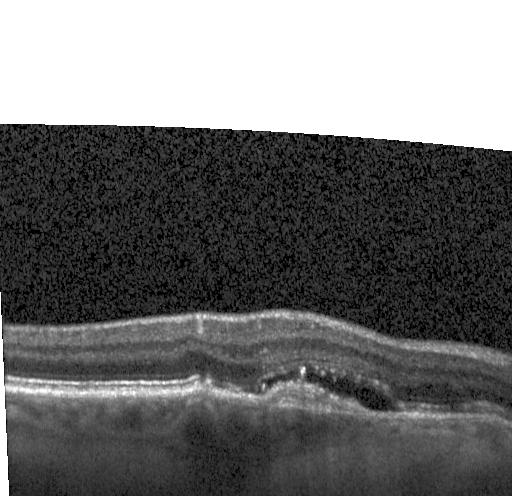

Macular OCT: a choroidal neovascular membrane.